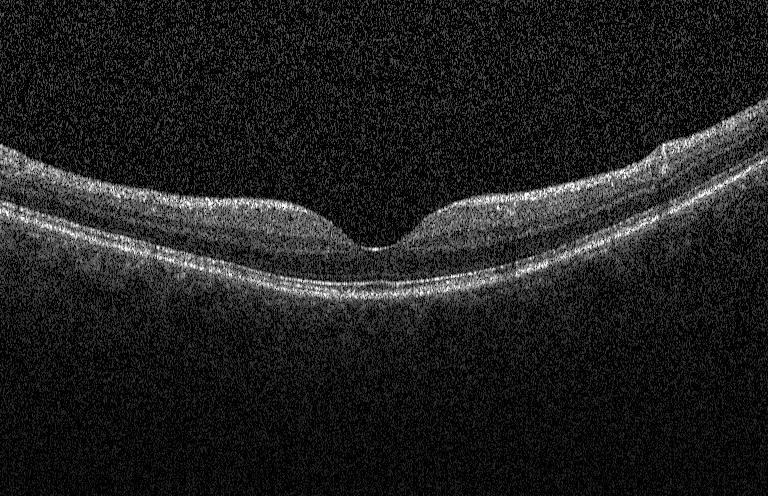

Optical coherence tomography B-scan. Centered on the fovea. Finding: neither choroidal neovascularization, diabetic macular edema, nor drusen.